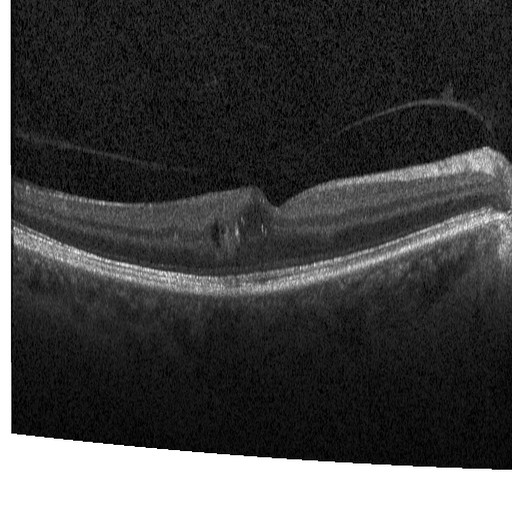 Macular OCT: DME.